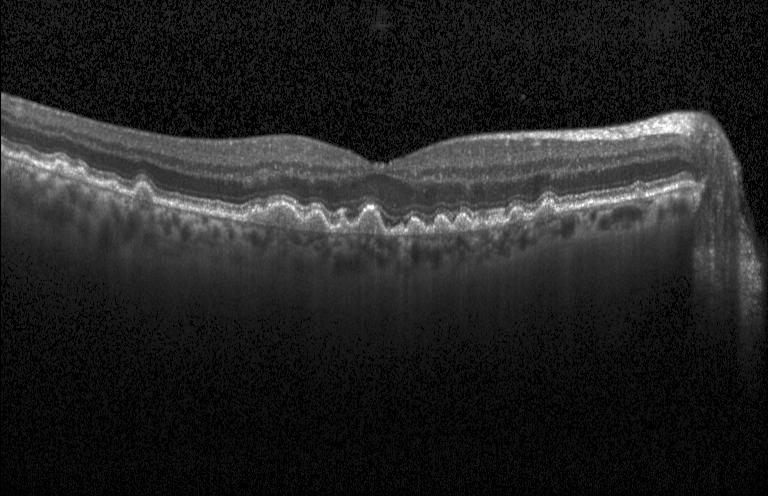
Fovea-centered, retinal OCT B-scan
Impression: sub-RPE drusenoid deposits.